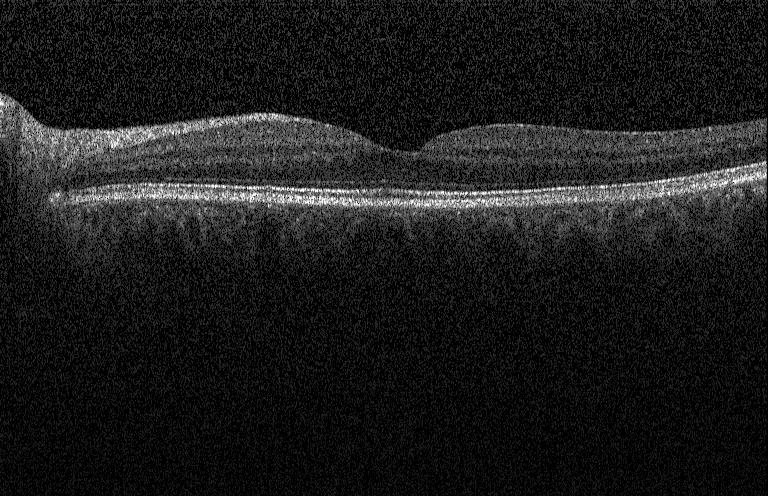 Diagnosis: neither choroidal neovascularization, diabetic macular edema, nor drusen.